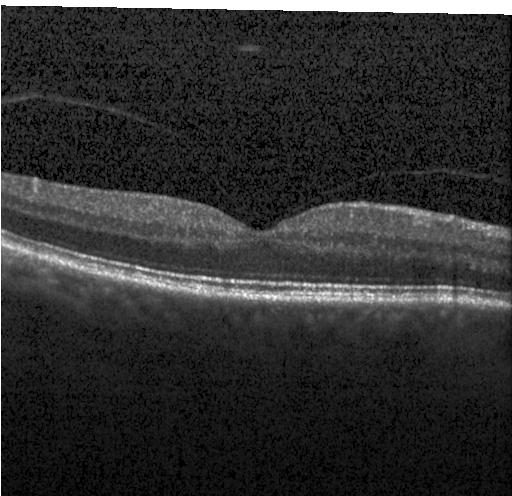
OCT line scan, instrument: Heidelberg Spectralis. Assessment: no choroidal neovascularization, diabetic macular edema, or drusen.